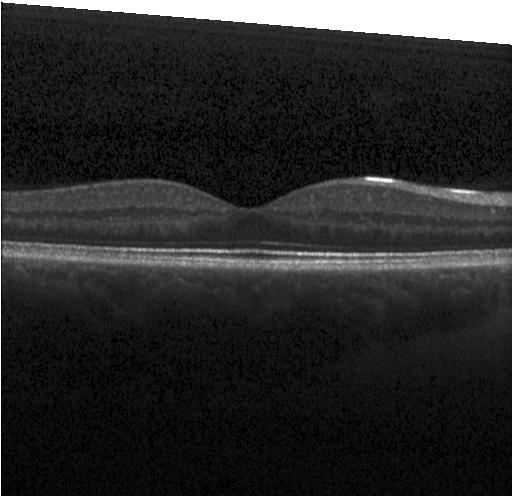
Diagnosis: no choroidal neovascularization, diabetic macular edema, or drusen.